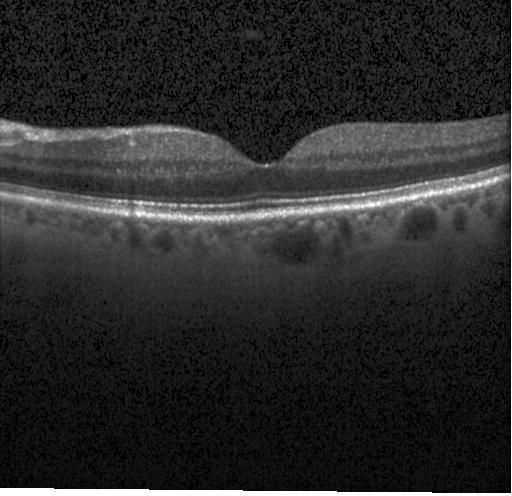

Finding: no choroidal neovascularization, no diabetic macular edema, and no drusen.